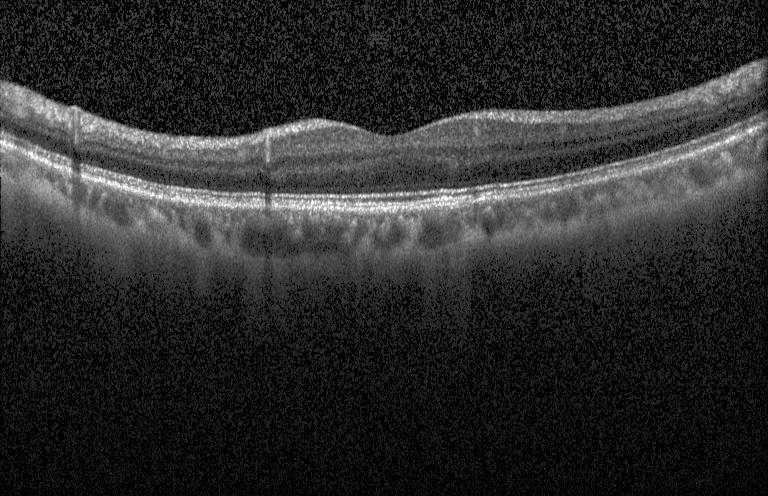

OCT finding: no evidence of CNV, DME, or drusen.